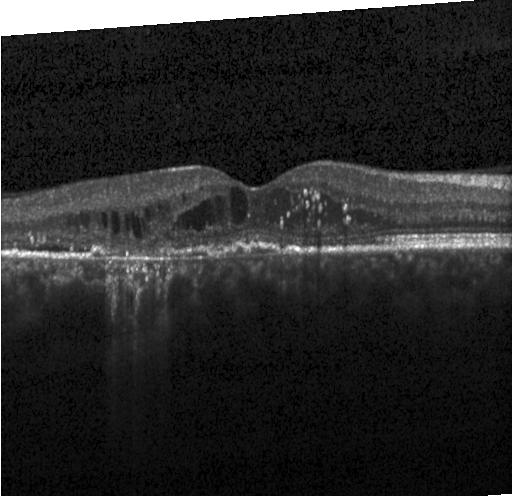
Retinal OCT cross-section; through the macula. This B-scan demonstrates CNV.